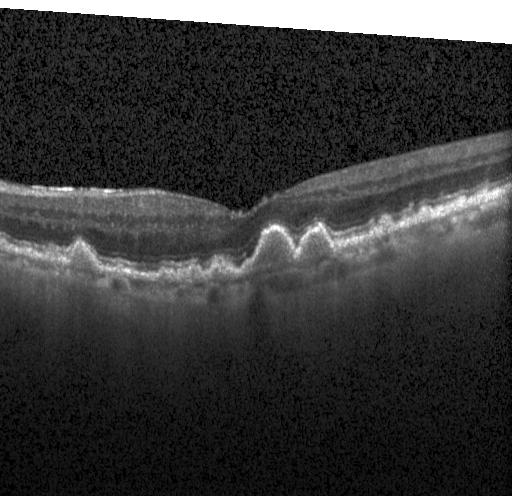
OCT finding: multiple drusen.